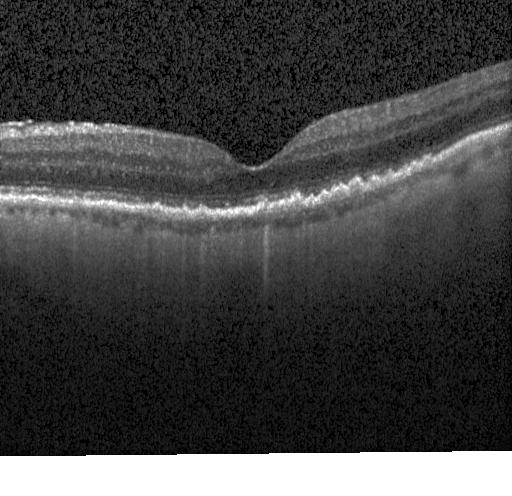 Optical coherence tomography B-scan. Heidelberg Spectralis OCT system.
Impression: multiple drusen.